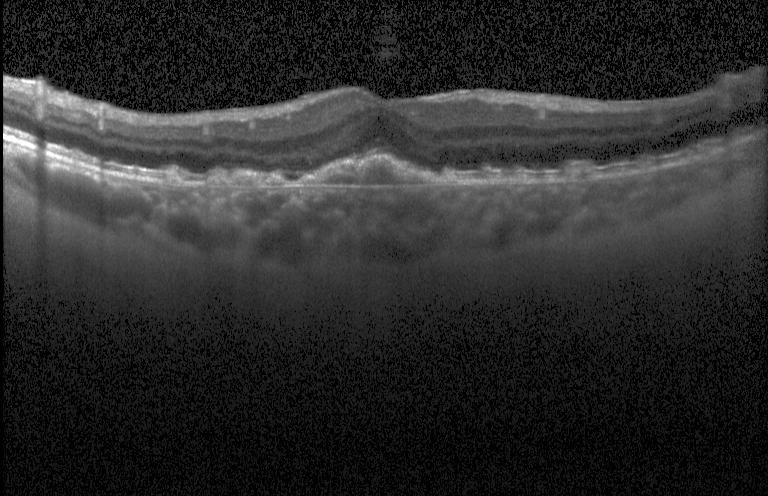

Finding: a choroidal neovascular membrane.